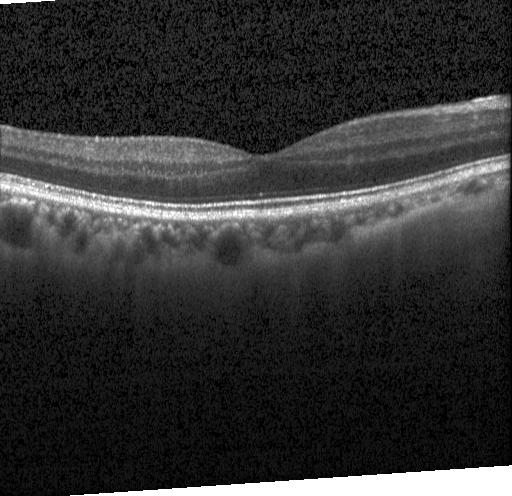

Dx: no evidence of choroidal neovascularization, diabetic macular edema, or drusen.